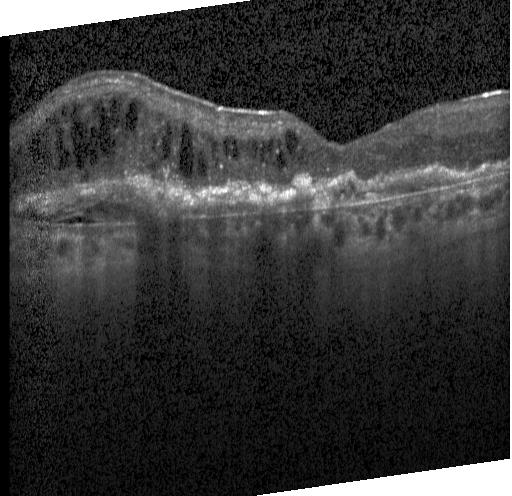 Macular OCT demonstrating CNV.